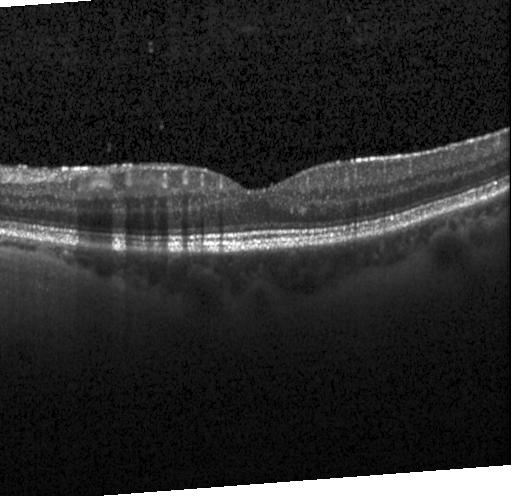
Optical coherence tomography scan. Macular scan. OCT finding: no choroidal neovascularization, diabetic macular edema, or drusen.